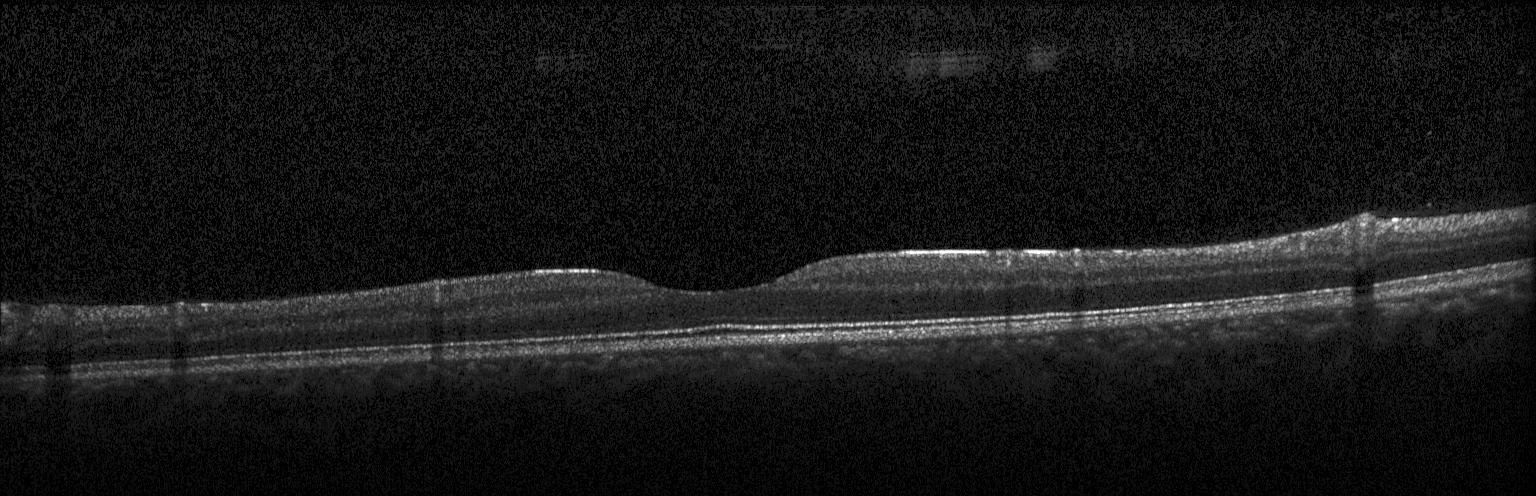

Impression: no choroidal neovascularization, no diabetic macular edema, and no drusen.